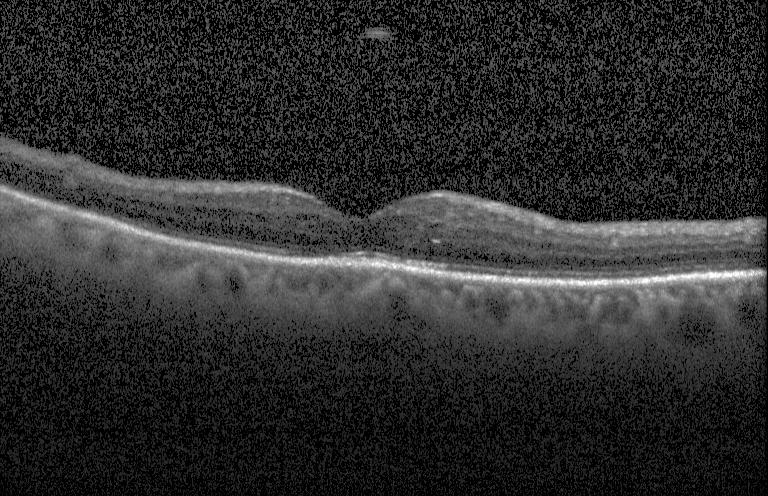
OCT line scan — Macular OCT: no CNV, DME, or drusen.